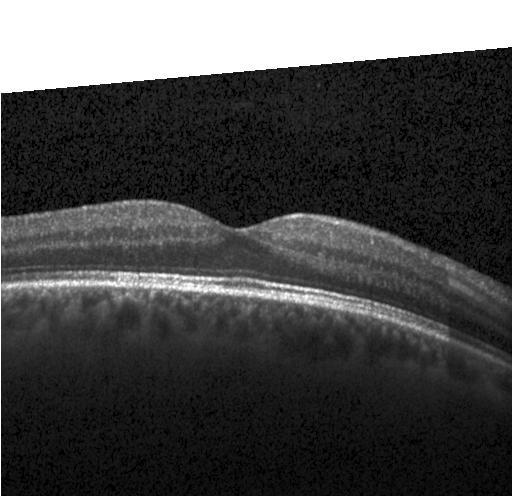

Spectral-domain OCT · Heidelberg Spectralis OCT system · horizontal scan through the fovea · OCT B-scan
OCT finding: no CNV, DME, or drusen.